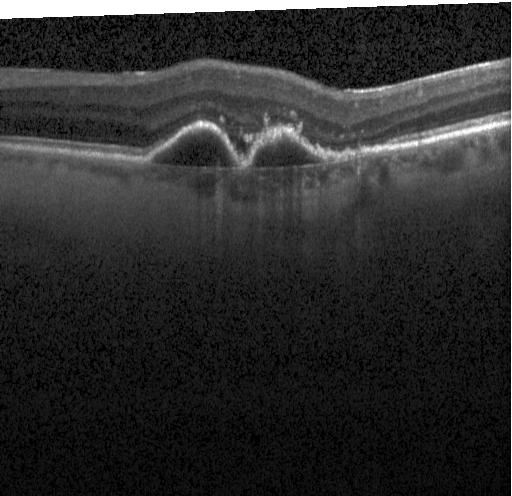
OCT finding: choroidal neovascularization (CNV).